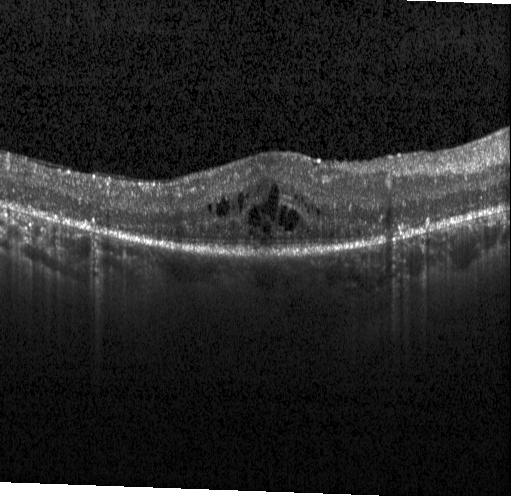

Diagnosis: DME.